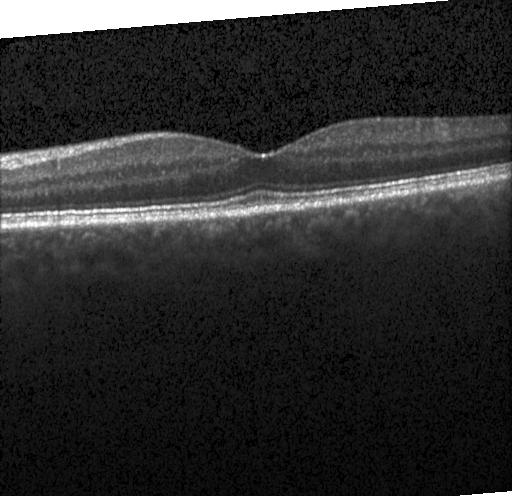 OCT B-scan. Macular OCT: no evidence of CNV, DME, or drusen.